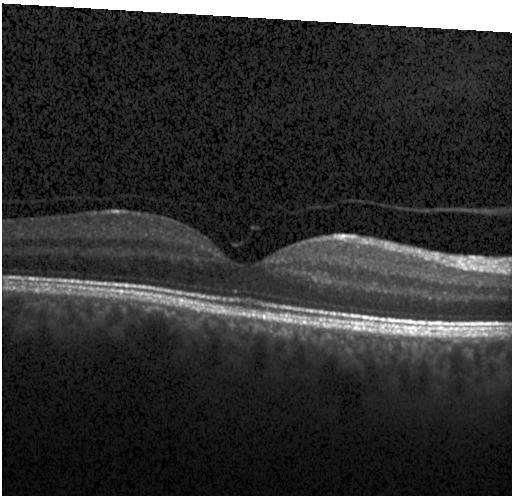
Spectral-domain OCT. Optical coherence tomography B-scan. Assessment: neither choroidal neovascularization, diabetic macular edema, nor drusen.